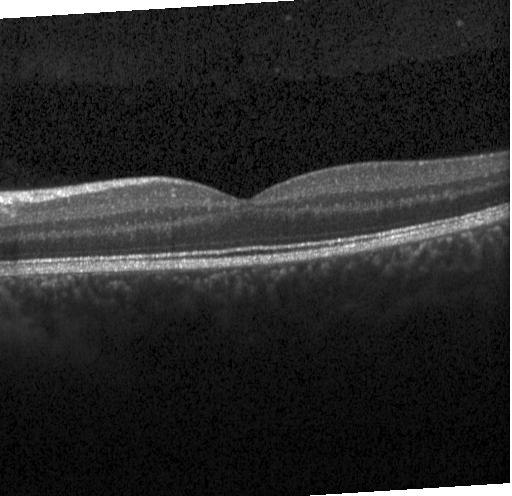

No CNV, DME, or drusen.